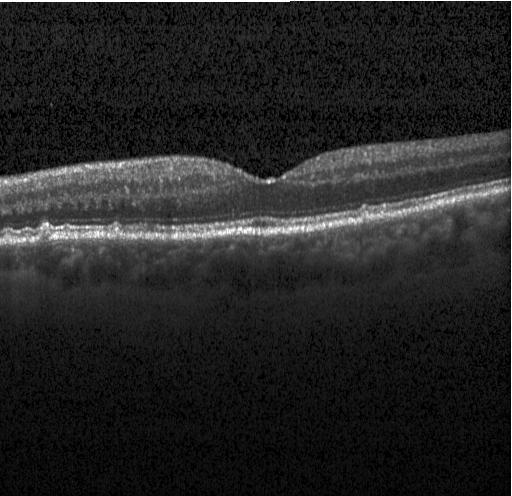 Instrument: Heidelberg Spectralis. Retinal OCT B-scan.
Impression: sub-RPE drusenoid deposits.